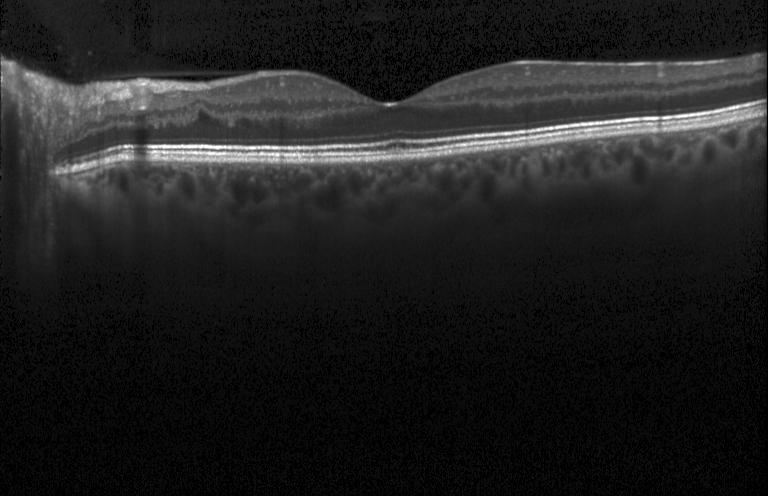
Finding: no choroidal neovascularization, diabetic macular edema, or drusen.